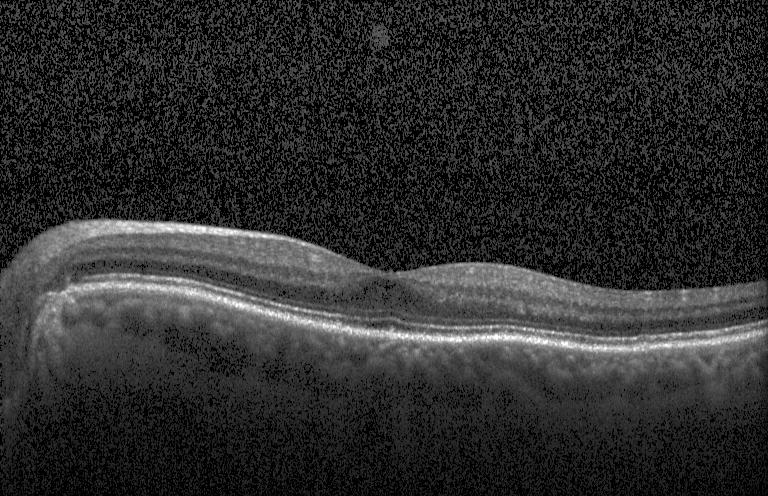
Retinal OCT B-scan · acquired on a Heidelberg Spectralis · through the macula · spectral-domain optical coherence tomography
Macular OCT: no evidence of choroidal neovascularization, diabetic macular edema, or drusen.